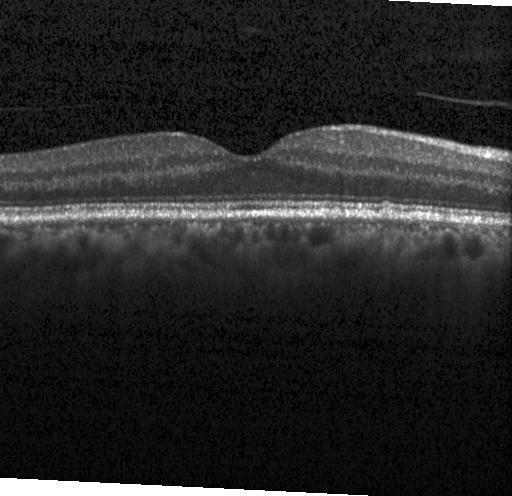

Diagnosis: neither choroidal neovascularization, diabetic macular edema, nor drusen.